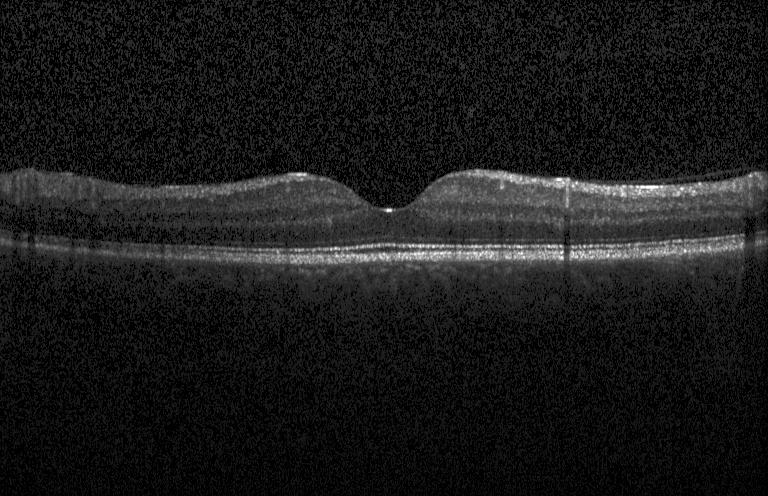
Dx: no CNV, no DME, and no drusen.